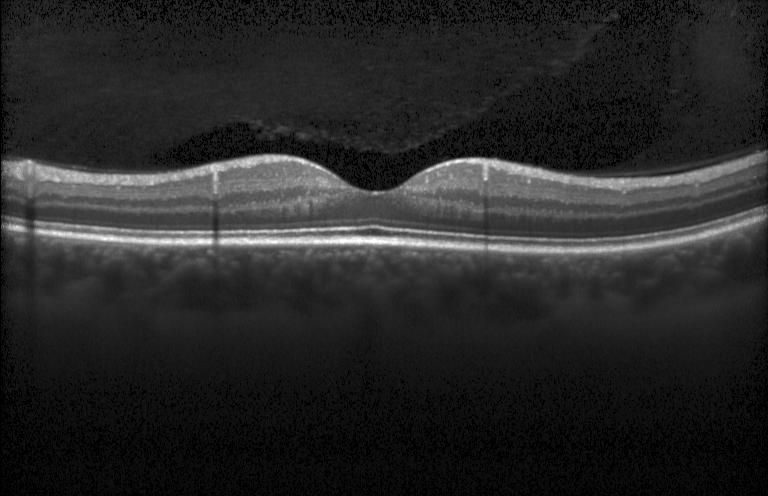
Retinal OCT cross-section showing no CNV, DME, or drusen.